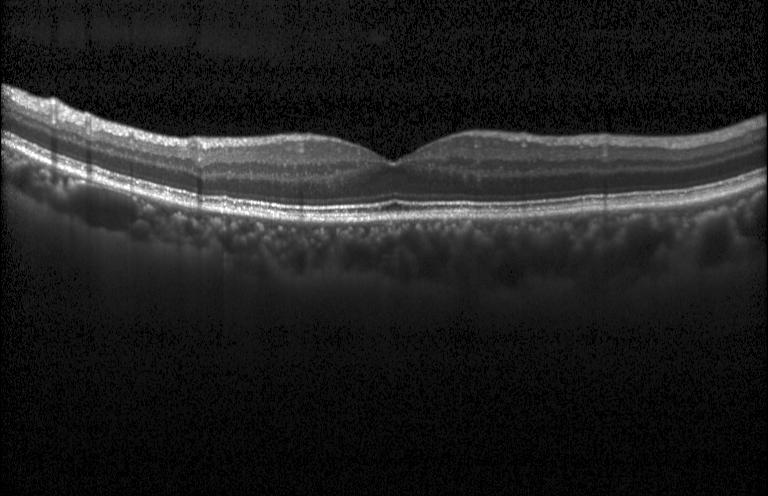

Spectral-domain optical coherence tomography. Instrument: Heidelberg Spectralis. Fovea-centered. Retinal OCT B-scan. Dx: neither choroidal neovascularization, diabetic macular edema, nor drusen.